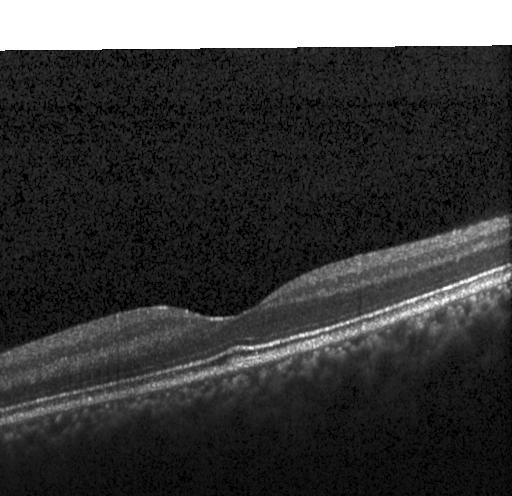
OCT B-scan; spectral-domain OCT; horizontal scan through the fovea; instrument: Heidelberg Spectralis. Dx: no evidence of choroidal neovascularization, diabetic macular edema, or drusen.